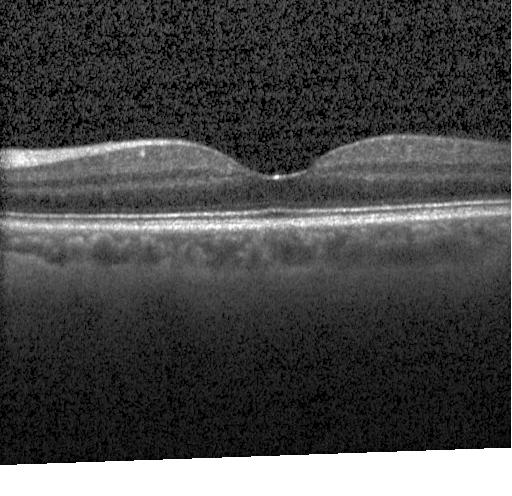

Acquired on a Heidelberg Spectralis; OCT B-scan; fovea-centered — This B-scan demonstrates neither choroidal neovascularization, diabetic macular edema, nor drusen.